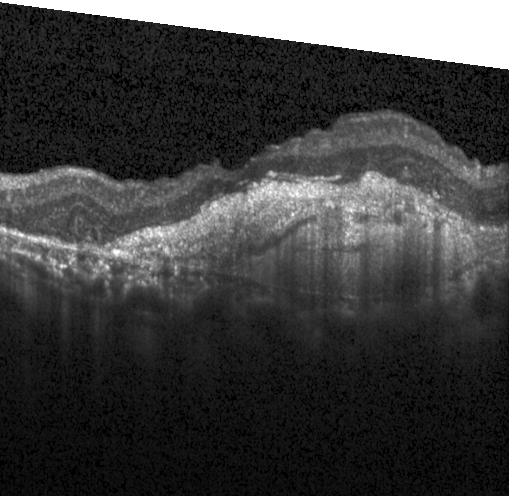
Diagnosis: a choroidal neovascular membrane.